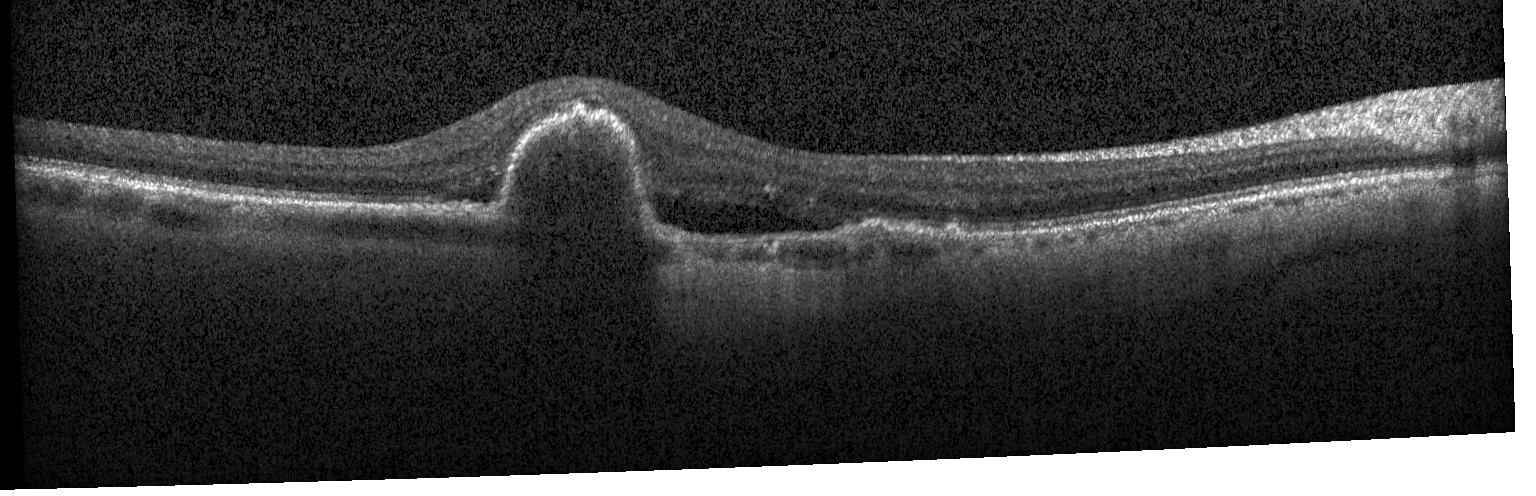
Centered on the fovea, OCT B-scan.
OCT finding: CNV.